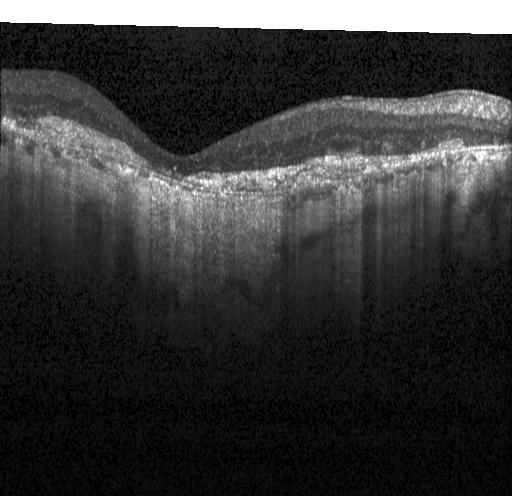 Macular OCT: CNV.